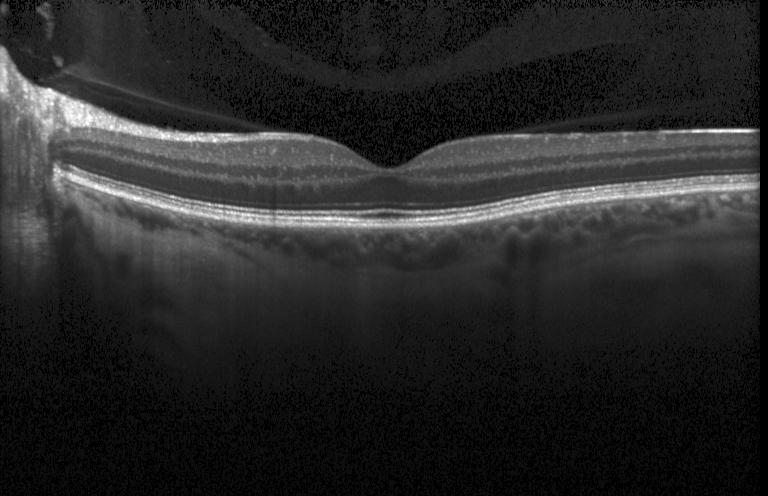

Optical coherence tomography B-scan — The scan shows no CNV, no DME, and no drusen.